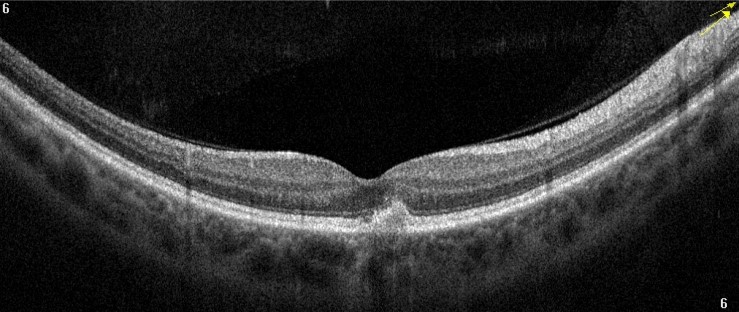

Spectral-domain OCT B-scan: age-related macular degeneration.